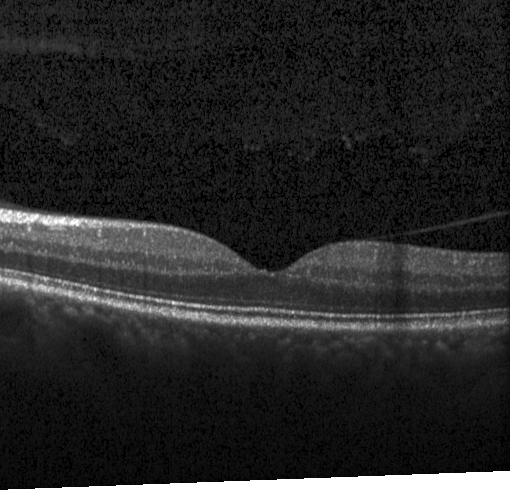 Optical coherence tomography scan; spectral-domain optical coherence tomography; horizontal scan through the fovea.
Macular OCT: no evidence of choroidal neovascularization, diabetic macular edema, or drusen.